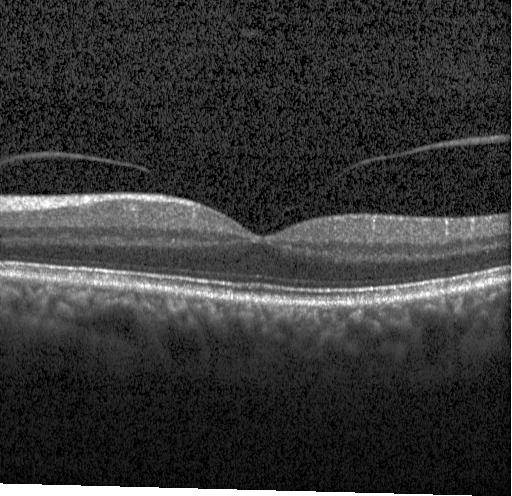
Optical coherence tomography scan
Diagnosis: no CNV, no DME, and no drusen.